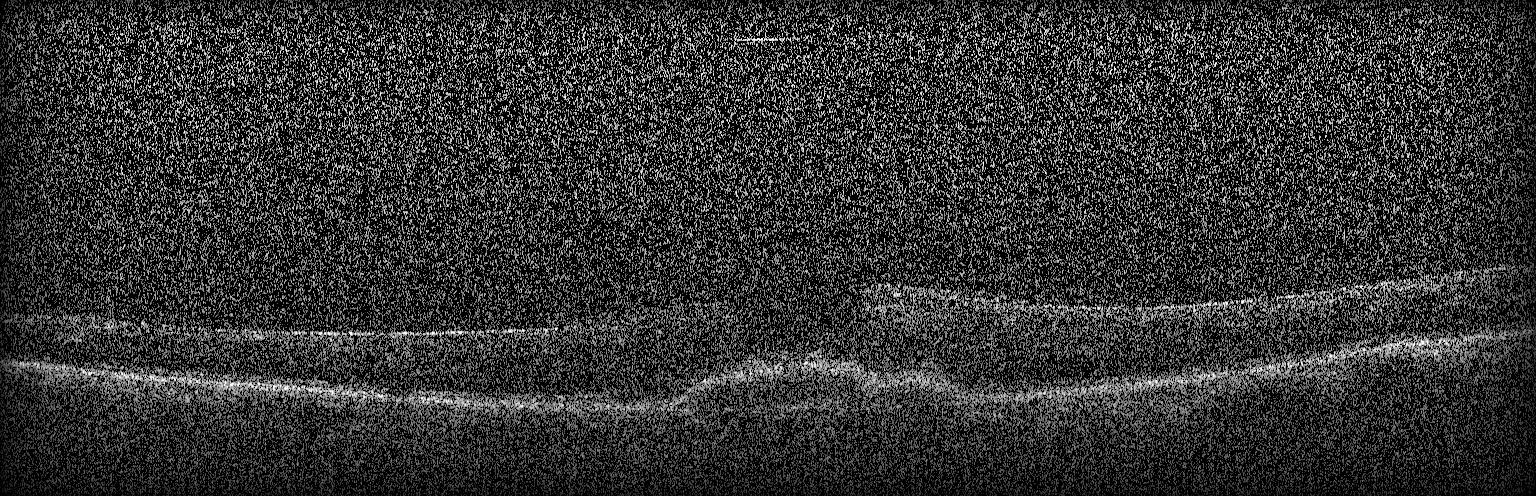 A choroidal neovascular membrane.